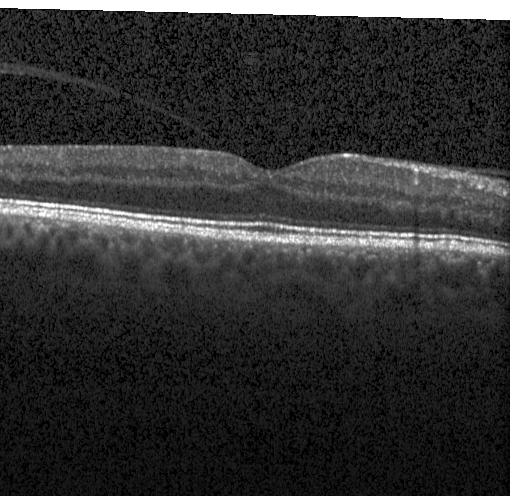
Optical coherence tomography scan; spectral-domain OCT; centered on the fovea; Heidelberg Spectralis.
Diagnosis: no choroidal neovascularization, no diabetic macular edema, and no drusen.